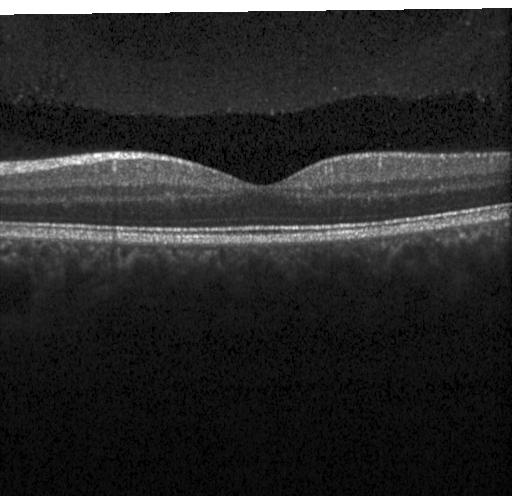

OCT finding: no evidence of choroidal neovascularization, diabetic macular edema, or drusen.